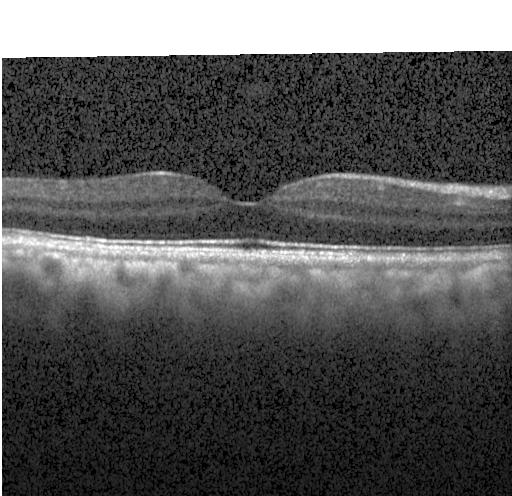
SD-OCT, retinal OCT cross-section, macular scan, instrument: Heidelberg Spectralis
This B-scan demonstrates no choroidal neovascularization, no diabetic macular edema, and no drusen.